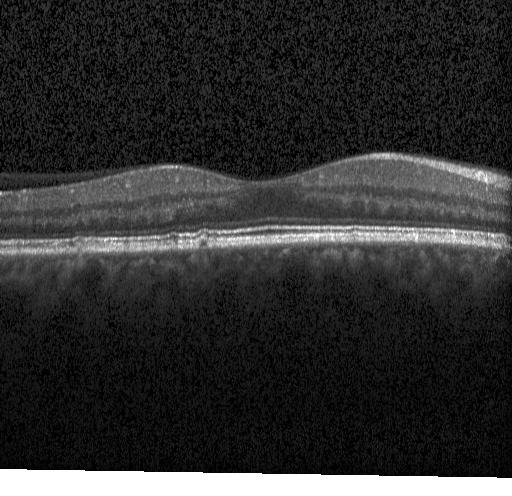
Dx: sub-RPE drusenoid deposits.